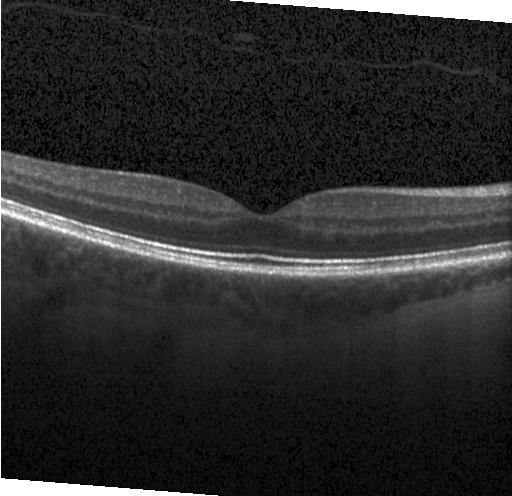
OCT line scan · Heidelberg Spectralis OCT system · spectral-domain optical coherence tomography — No choroidal neovascularization, diabetic macular edema, or drusen.